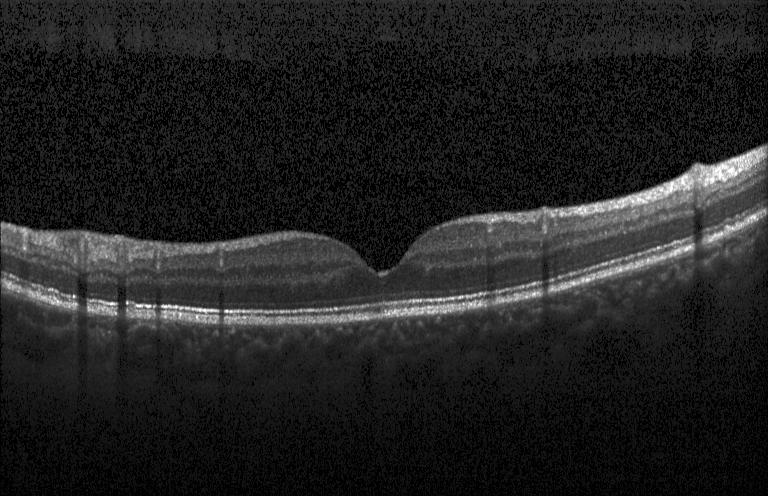 Diagnosis: no evidence of choroidal neovascularization, diabetic macular edema, or drusen.